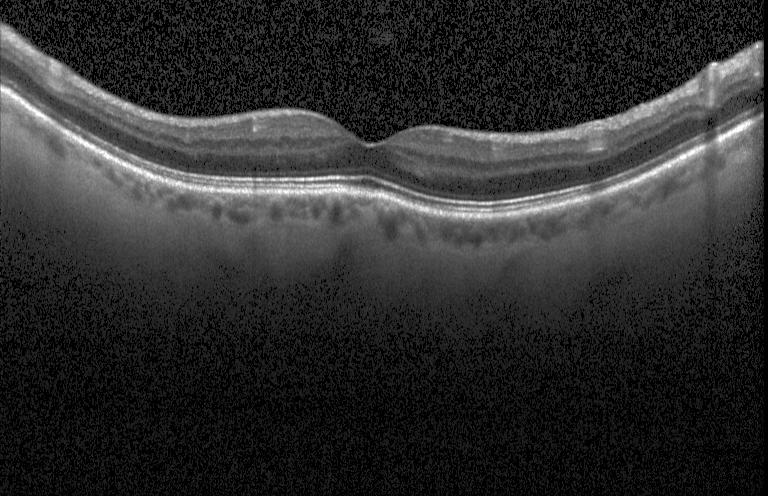
Spectral-domain OCT. OCT line scan. Heidelberg Spectralis OCT system. Macular OCT: no evidence of choroidal neovascularization, diabetic macular edema, or drusen.